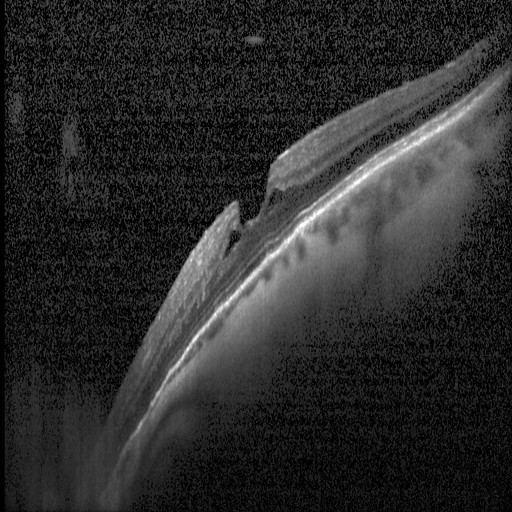 Assessment: DME.